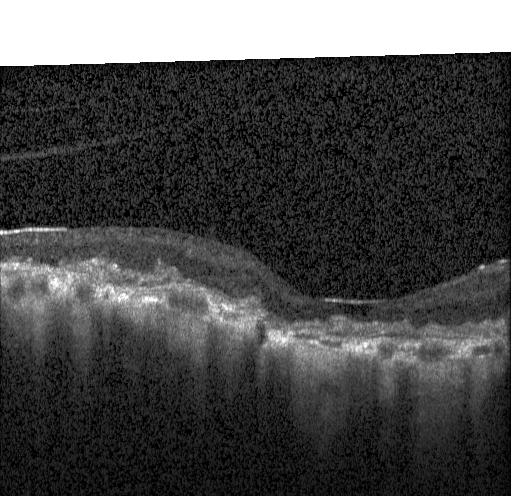 Optical coherence tomography scan. Horizontal scan through the fovea. Spectral-domain OCT. Acquired on a Heidelberg Spectralis — Macular OCT: a choroidal neovascular membrane.